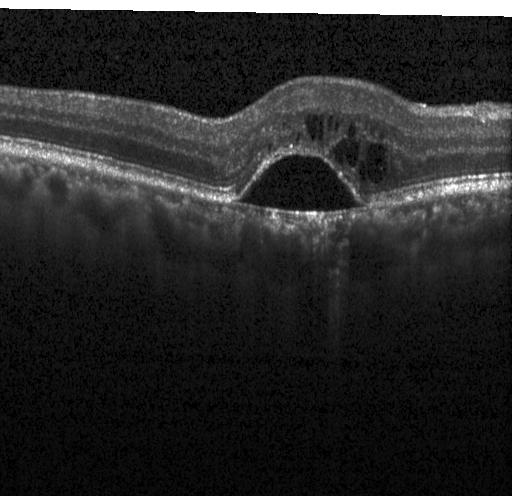 Fovea-centered. Optical coherence tomography scan. Acquired on a Heidelberg Spectralis. Choroidal neovascularization (CNV).